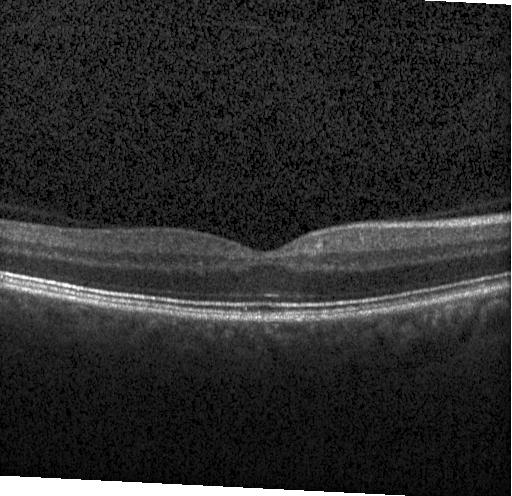
Optical coherence tomography scan, through the macula, spectral-domain OCT, instrument: Heidelberg Spectralis. Impression: neither CNV, DME, nor drusen.